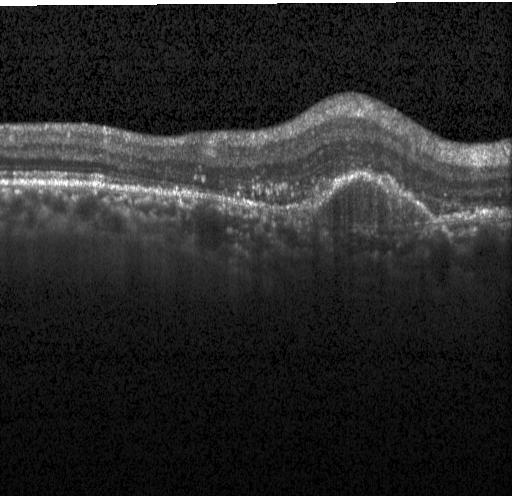

Assessment: choroidal neovascularization.